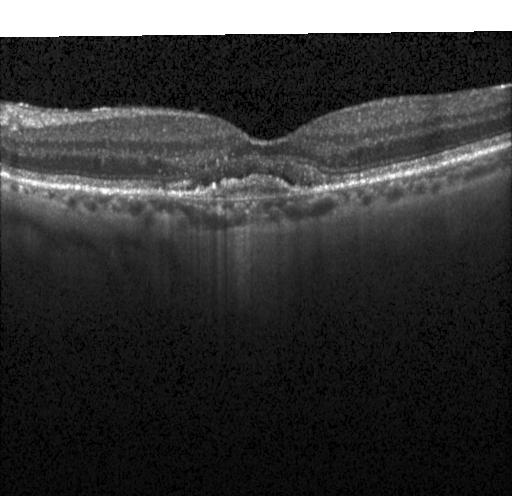
Optical coherence tomography B-scan, centered on the fovea — Finding: choroidal neovascularization.